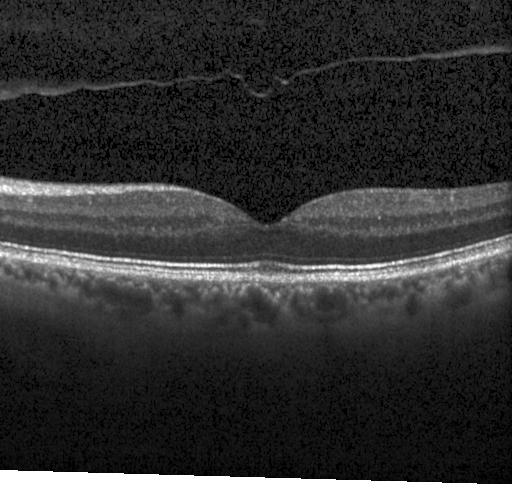 SD-OCT; acquired on a Heidelberg Spectralis; OCT B-scan — This B-scan demonstrates no choroidal neovascularization, diabetic macular edema, or drusen.